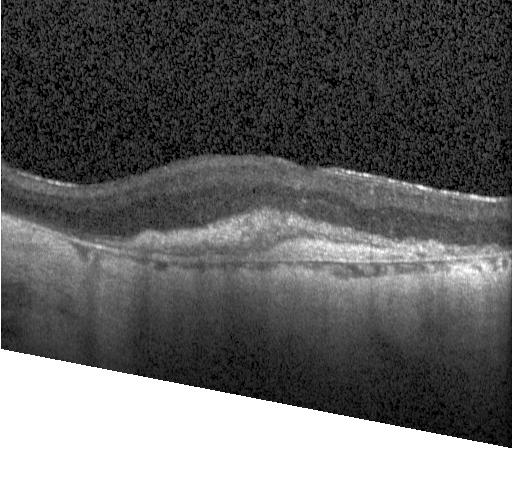 Optical coherence tomography B-scan. Horizontal scan through the fovea. Heidelberg Spectralis OCT system.
Finding: a choroidal neovascular membrane.